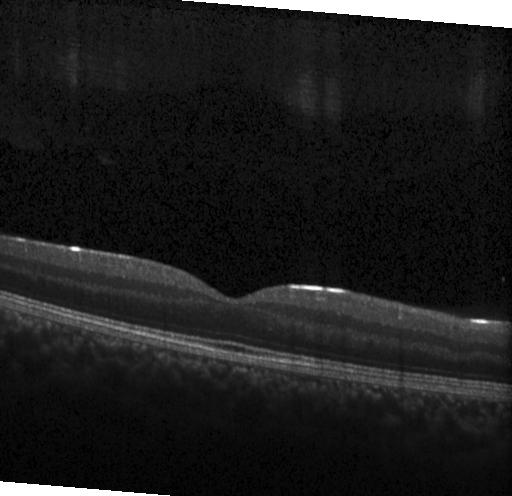
Fovea-centered · spectral-domain OCT · optical coherence tomography B-scan — Impression: no choroidal neovascularization, no diabetic macular edema, and no drusen.